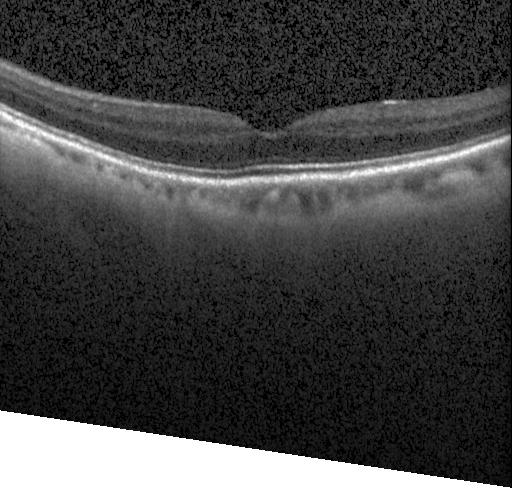
Heidelberg Spectralis. OCT B-scan. Spectral-domain OCT. Through the macula
Macular OCT: neither choroidal neovascularization, diabetic macular edema, nor drusen.